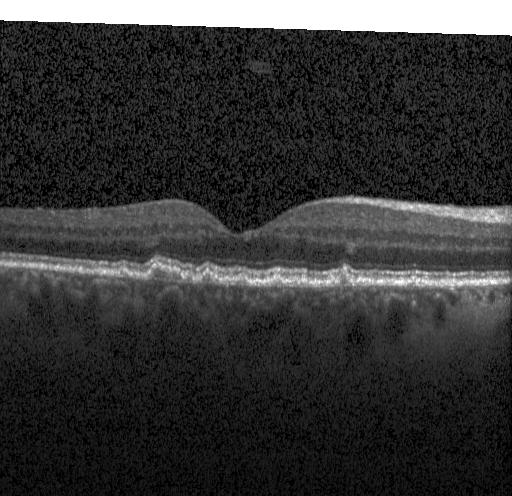

Spectral-domain OCT, Heidelberg Spectralis, retinal OCT B-scan
Impression: drusen.